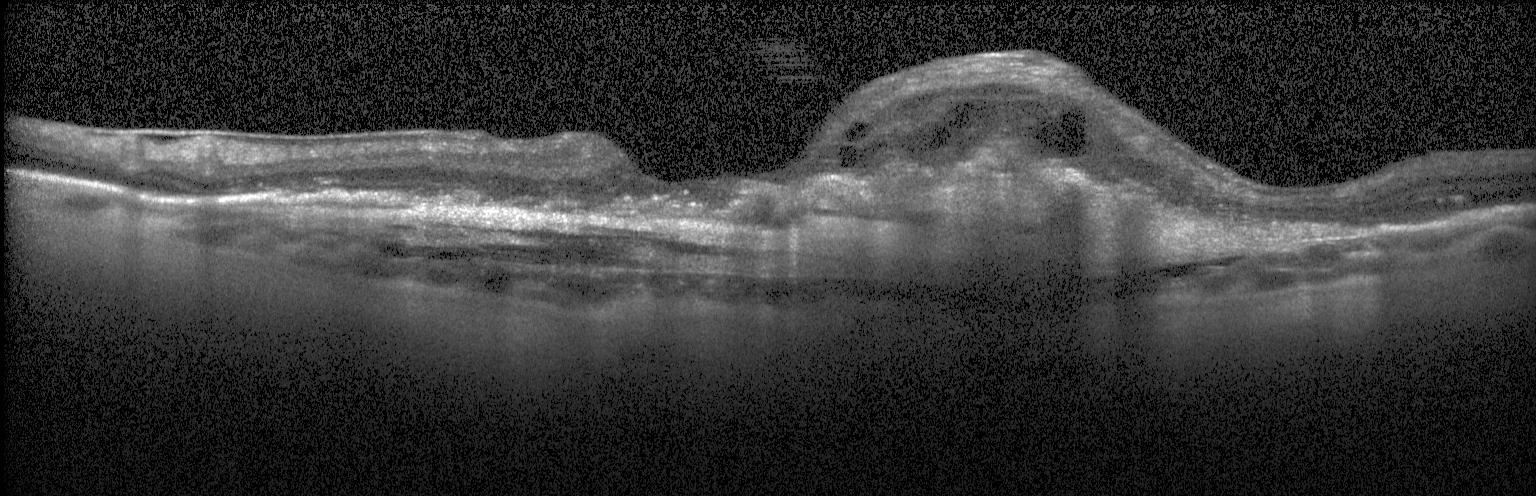 A choroidal neovascular membrane.